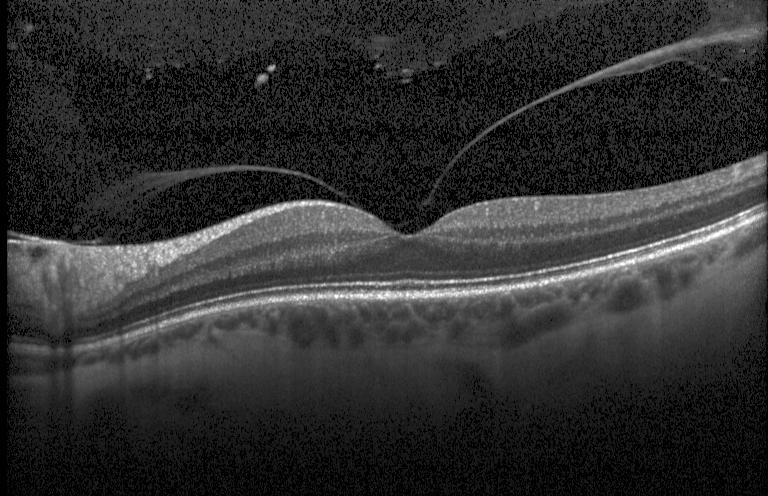

Heidelberg Spectralis OCT system; through the macula; OCT B-scan.
The scan shows no evidence of choroidal neovascularization, diabetic macular edema, or drusen.